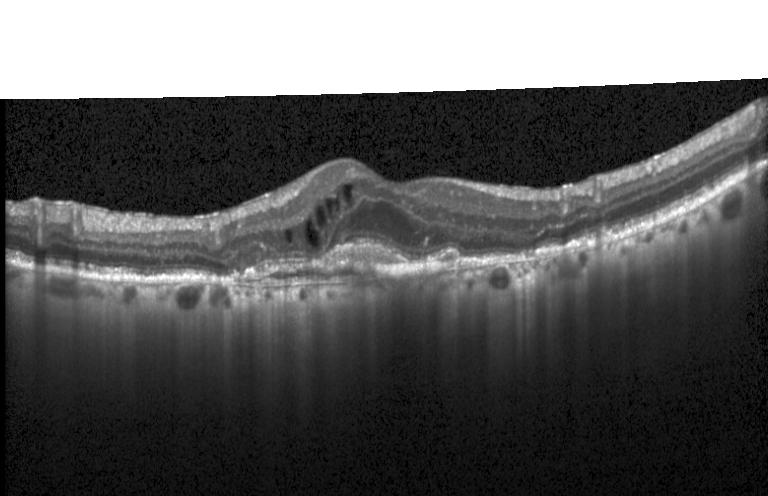

Retinal OCT B-scan · spectral-domain optical coherence tomography — The scan shows choroidal neovascularization (CNV).